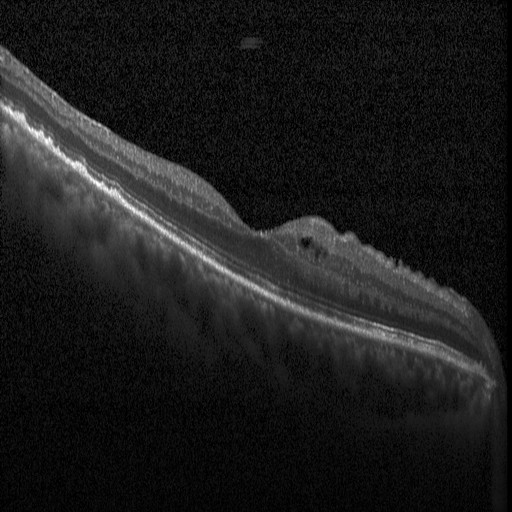

OCT finding: diabetic macular edema.